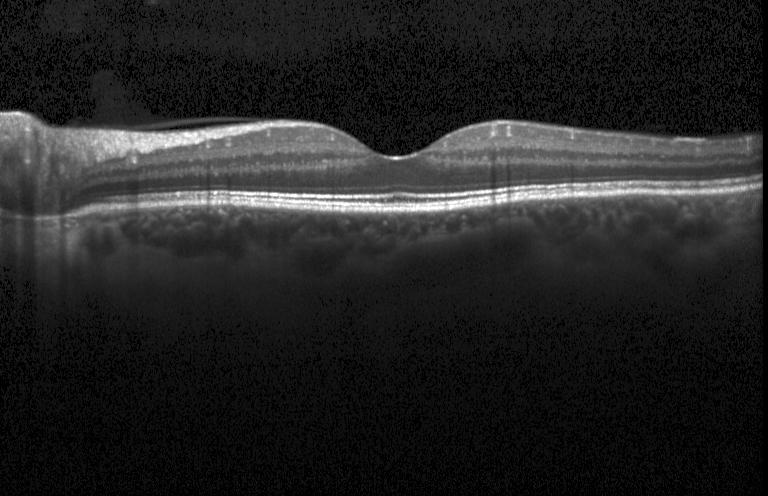
SD-OCT. OCT B-scan. Instrument: Heidelberg Spectralis. Fovea-centered.
No choroidal neovascularization, diabetic macular edema, or drusen.